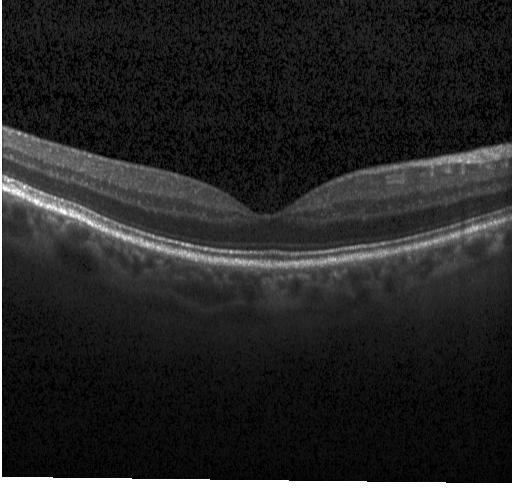 OCT line scan · acquired on a Heidelberg Spectralis
No CNV, no DME, and no drusen.